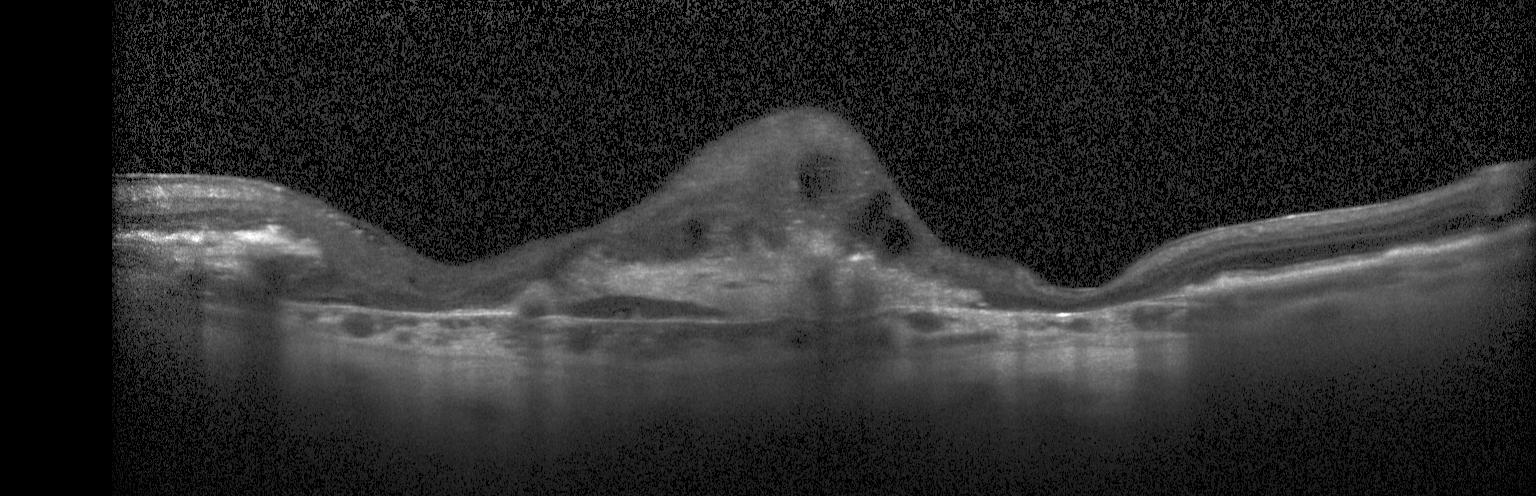 Diagnosis: a choroidal neovascular membrane.